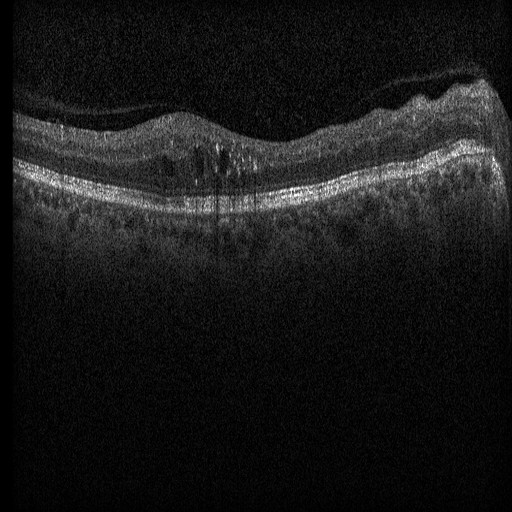 Fovea-centered, retinal OCT cross-section. Impression: diabetic macular edema (DME).